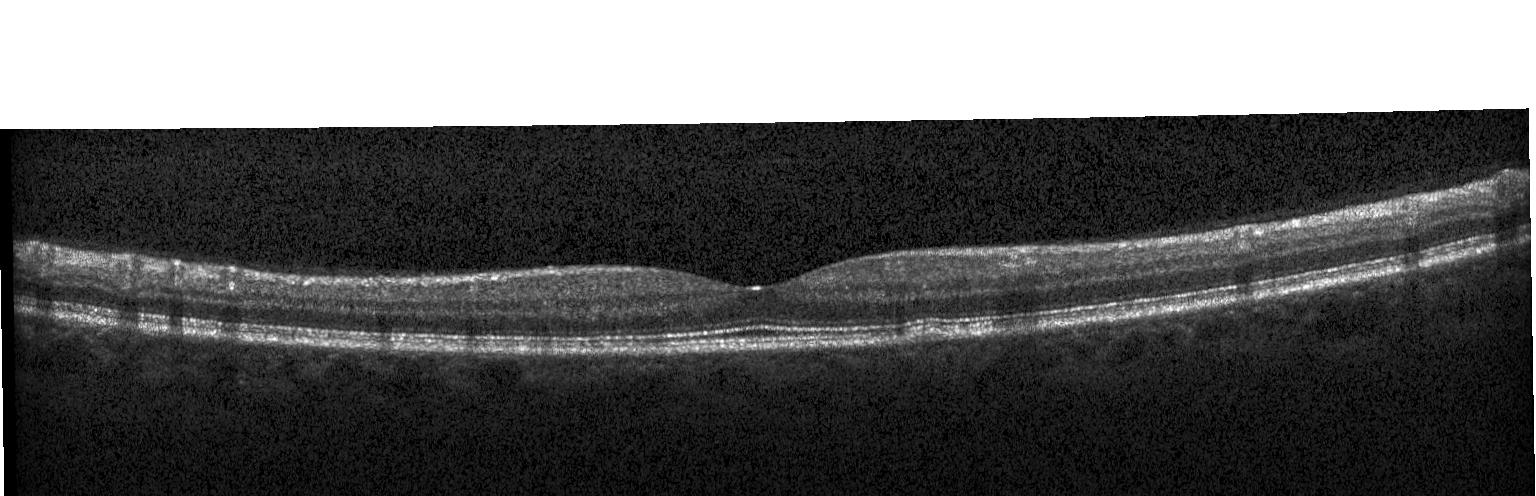
Retinal OCT cross-section; Heidelberg Spectralis. Impression: no evidence of choroidal neovascularization, diabetic macular edema, or drusen.